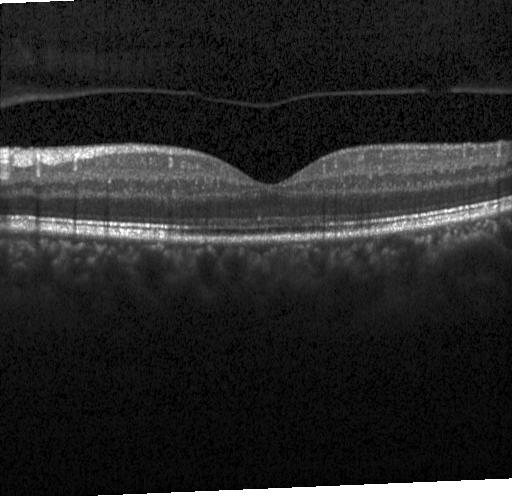

Horizontal scan through the fovea · optical coherence tomography scan · spectral-domain OCT · Heidelberg Spectralis OCT system.
Impression: no choroidal neovascularization, diabetic macular edema, or drusen.